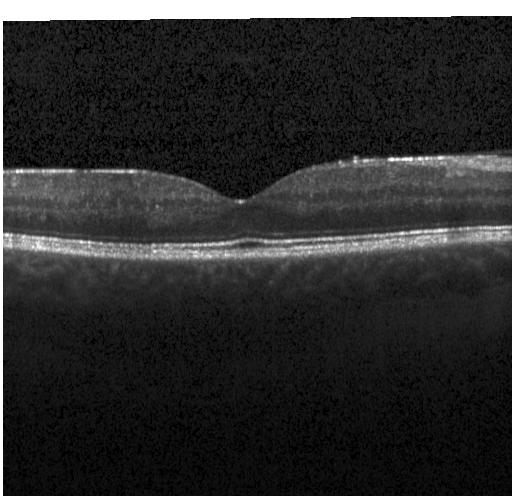 Impression: no choroidal neovascularization, no diabetic macular edema, and no drusen.